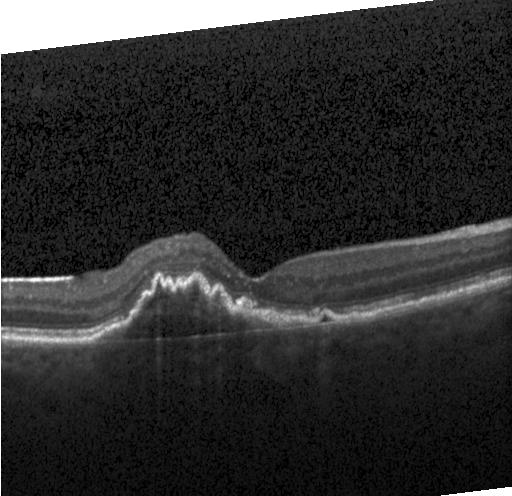 Retinal OCT cross-section.
Choroidal neovascularization.